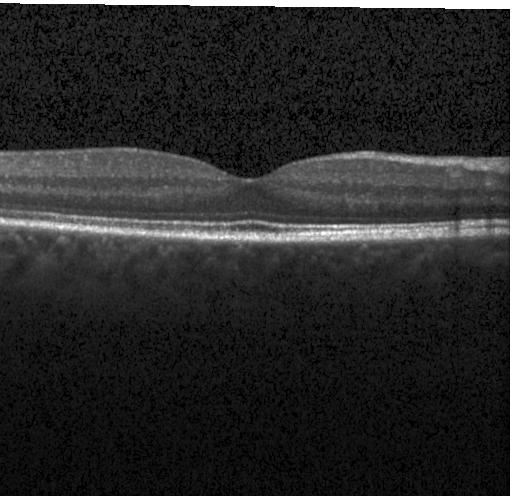
Macular scan. Retinal OCT cross-section.
Macular OCT: no CNV, DME, or drusen.